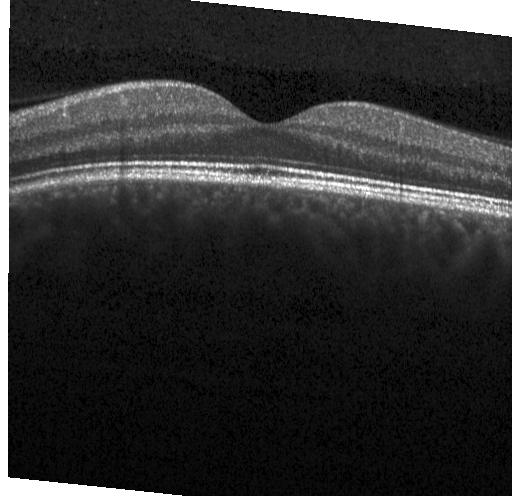
OCT finding: no CNV, DME, or drusen.